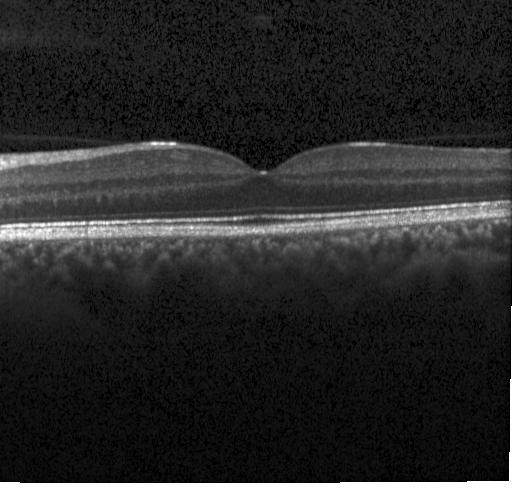 Impression: neither choroidal neovascularization, diabetic macular edema, nor drusen.